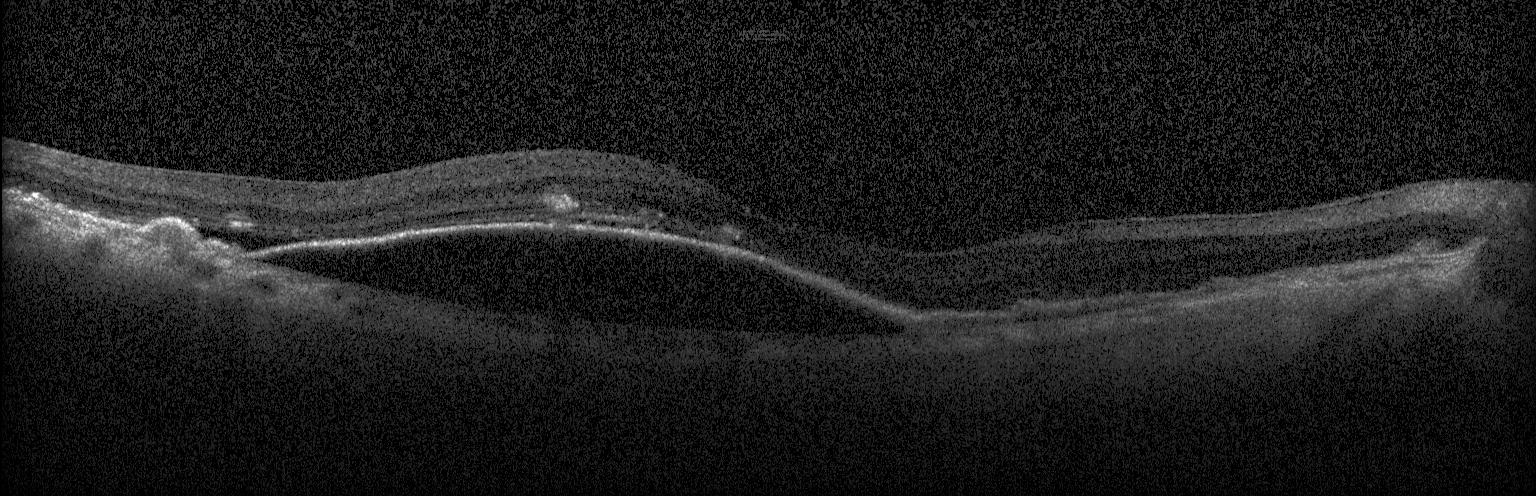
SD-OCT. Retinal OCT B-scan — Macular OCT: choroidal neovascularization (CNV).